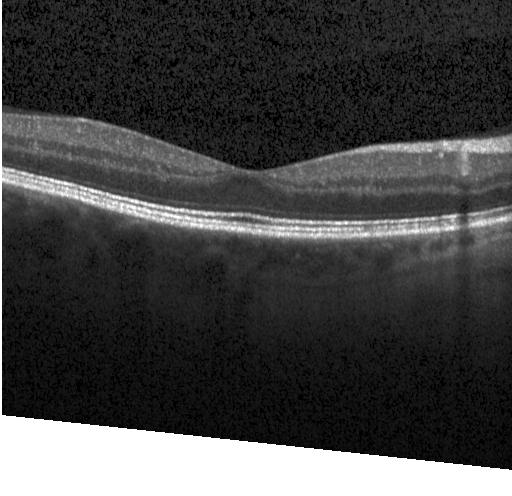
Through the macula. Acquired on a Heidelberg Spectralis. Spectral-domain OCT. Optical coherence tomography B-scan. Diagnosis: no CNV, DME, or drusen.